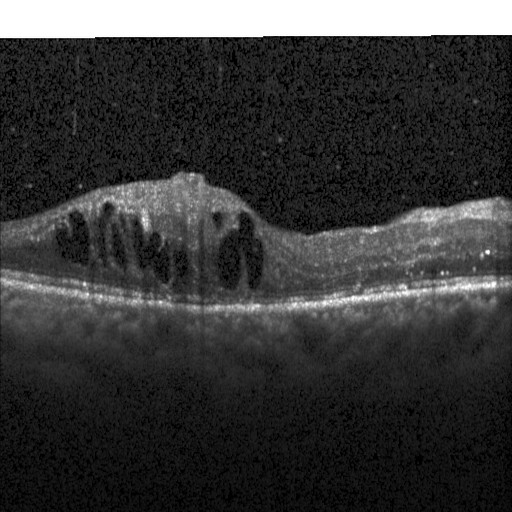
OCT line scan — Assessment: diabetic macular edema (DME).